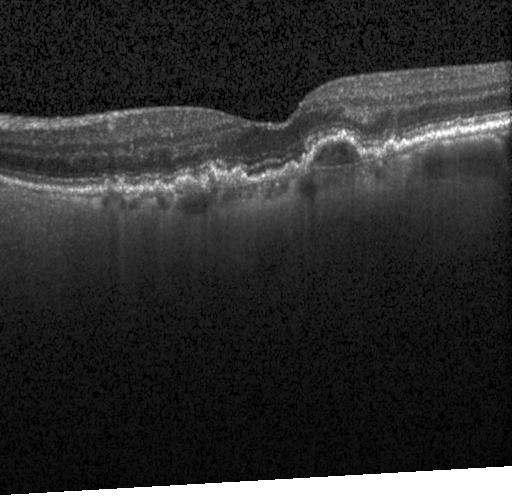
Spectral-domain OCT B-scan: CNV.